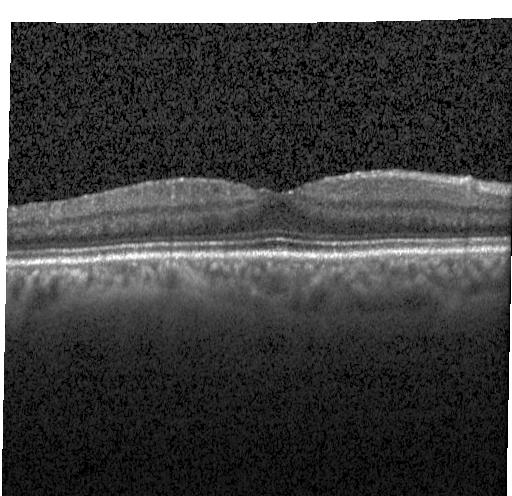 OCT line scan
Finding: no CNV, DME, or drusen.